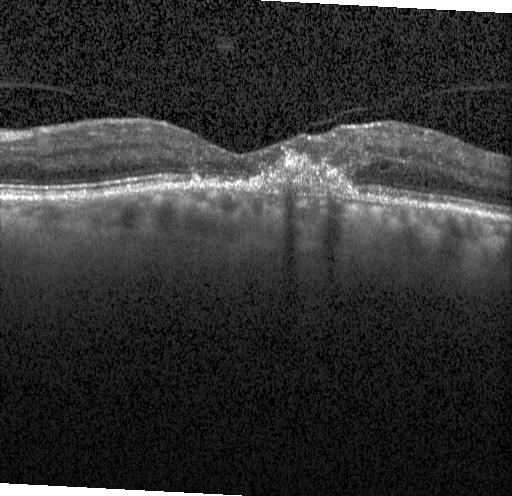 Instrument: Heidelberg Spectralis. Retinal OCT cross-section. Through the macula. Diagnosis: a choroidal neovascular membrane.